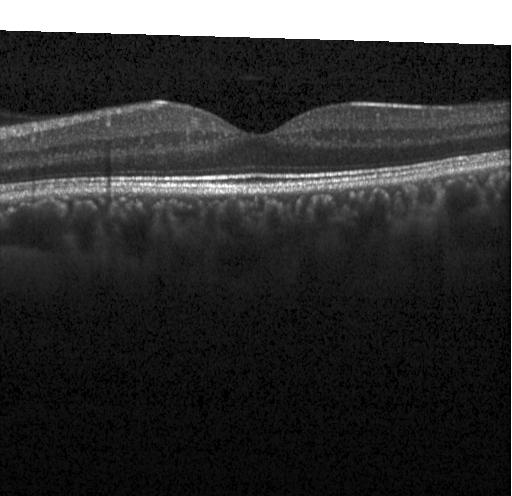 Dx: no choroidal neovascularization, diabetic macular edema, or drusen.